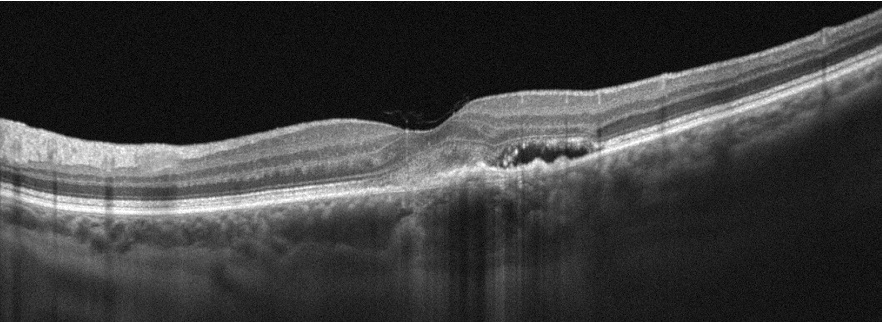 Optical coherence tomography scan. Finding: age-related macular degeneration (AMD).